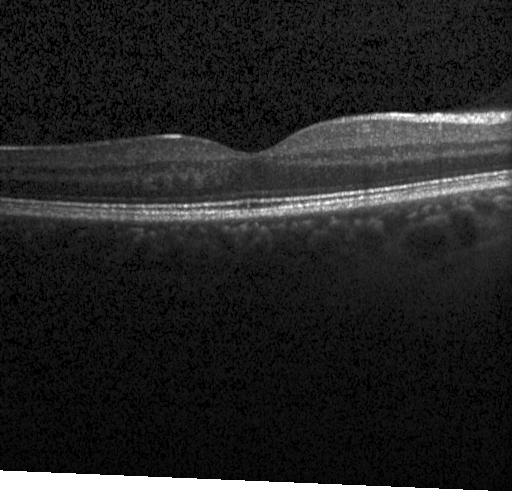

Optical coherence tomography B-scan. Diagnosis: no evidence of choroidal neovascularization, diabetic macular edema, or drusen.